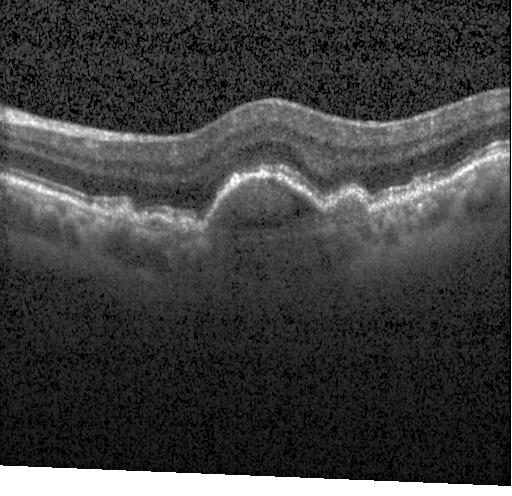 Retinal OCT B-scan; horizontal scan through the fovea
The scan shows multiple drusen.